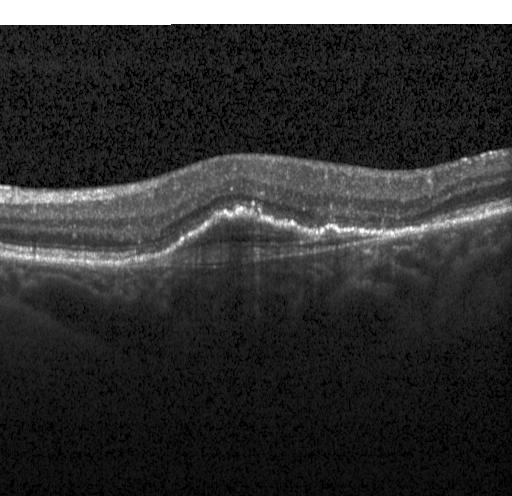

OCT B-scan showing choroidal neovascularization.